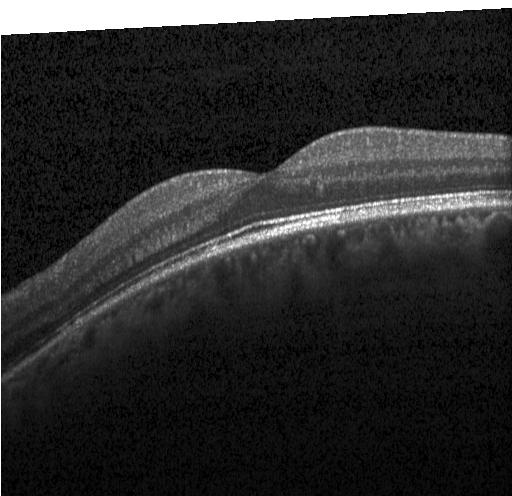

Spectral-domain optical coherence tomography · retinal OCT B-scan. OCT finding: neither choroidal neovascularization, diabetic macular edema, nor drusen.